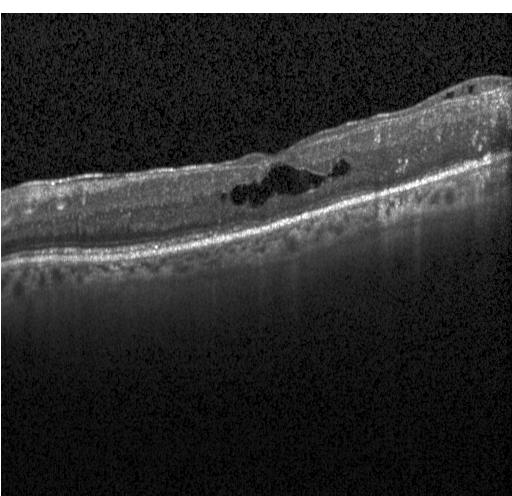
OCT finding: diabetic macular edema.